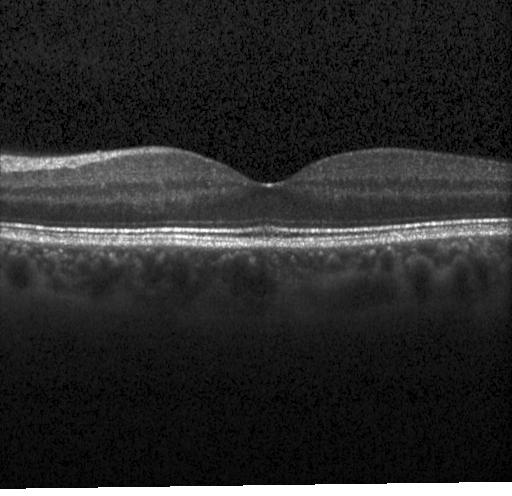

Macular OCT demonstrating no choroidal neovascularization, diabetic macular edema, or drusen.